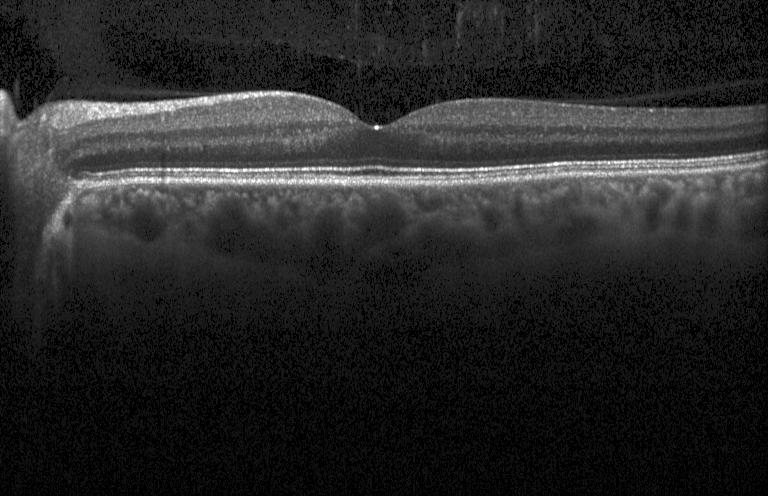

Dx: no choroidal neovascularization, diabetic macular edema, or drusen.